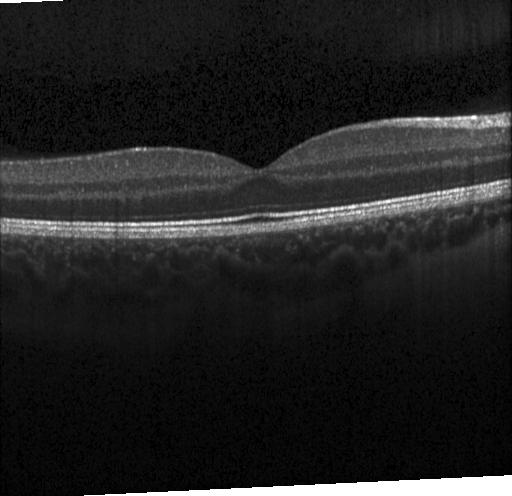 OCT B-scan
OCT finding: neither CNV, DME, nor drusen.